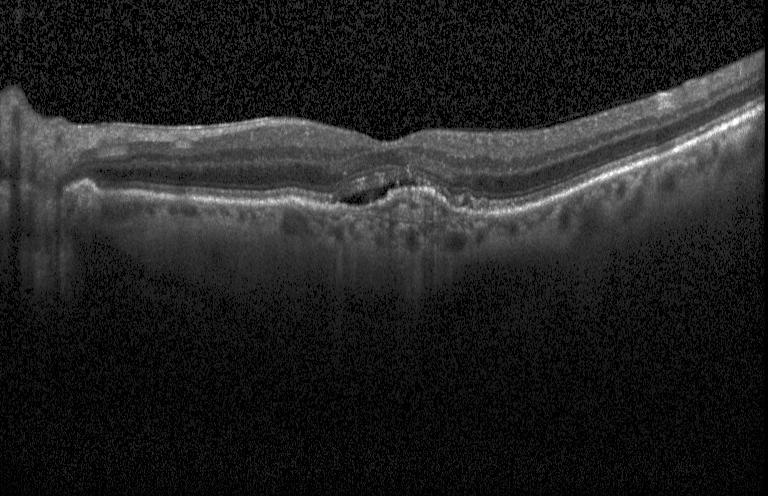 Retinal OCT cross-section
OCT finding: choroidal neovascularization (CNV).